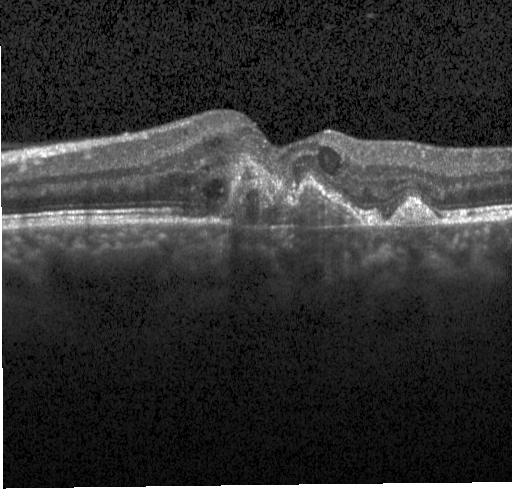

OCT finding: choroidal neovascularization.